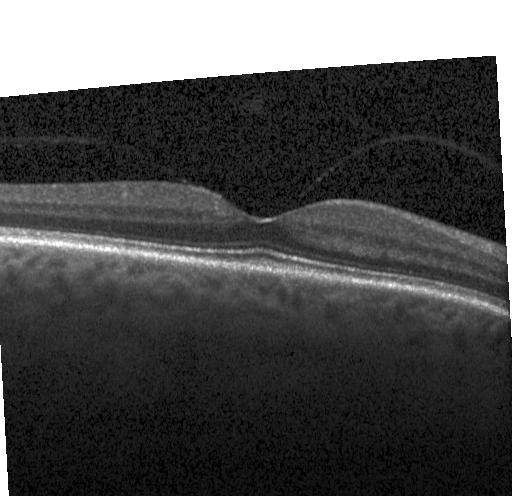 OCT B-scan; instrument: Heidelberg Spectralis; macular scan — Macular OCT: neither CNV, DME, nor drusen.